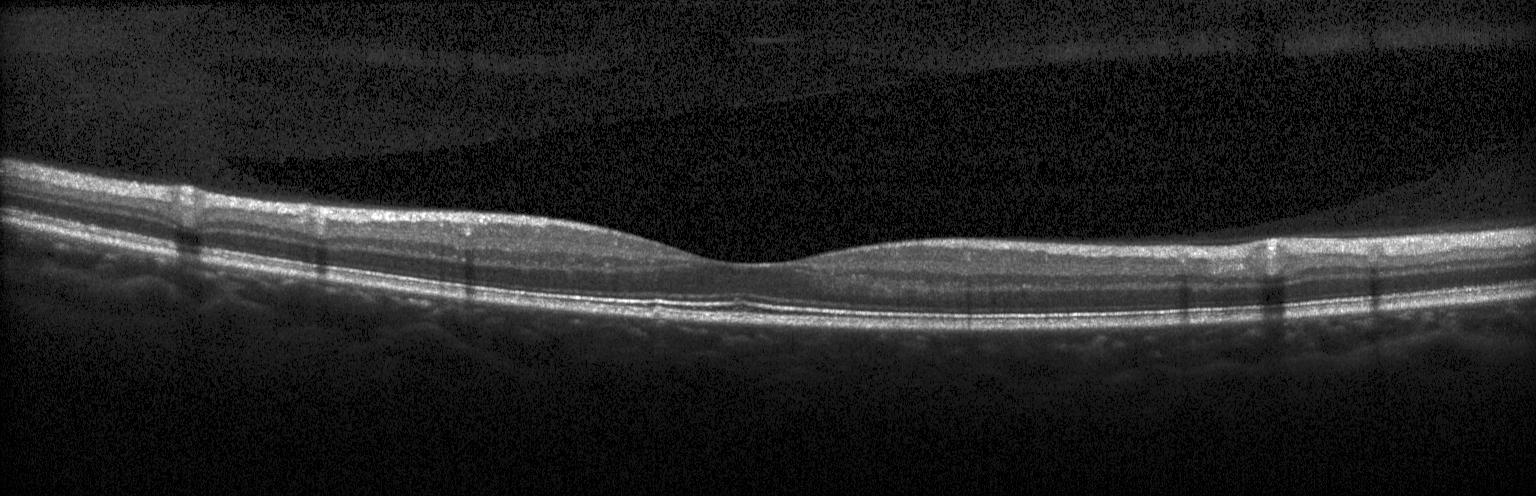

Heidelberg Spectralis OCT system, OCT B-scan, fovea-centered, spectral-domain OCT. Diagnosis: no evidence of CNV, DME, or drusen.